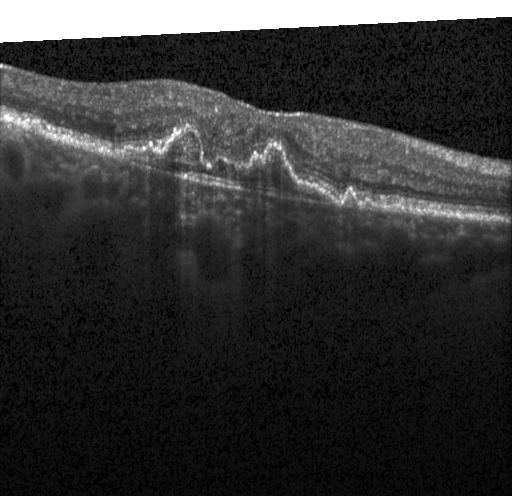
Spectral-domain OCT; retinal OCT cross-section.
OCT finding: CNV.